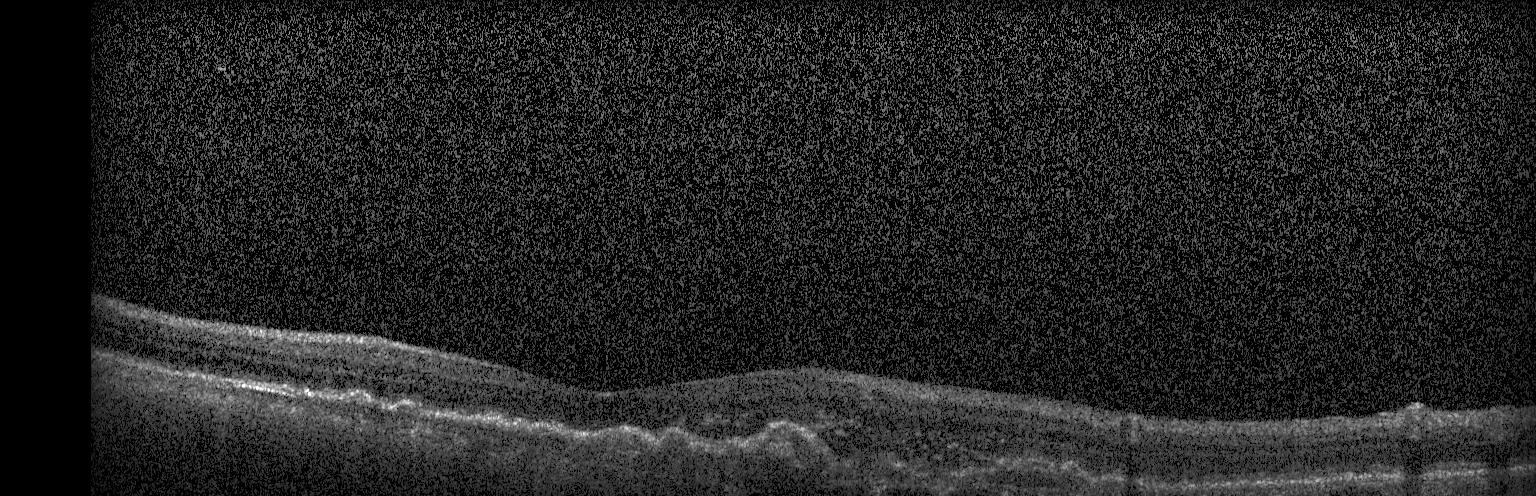
OCT line scan — Finding: a choroidal neovascular membrane.